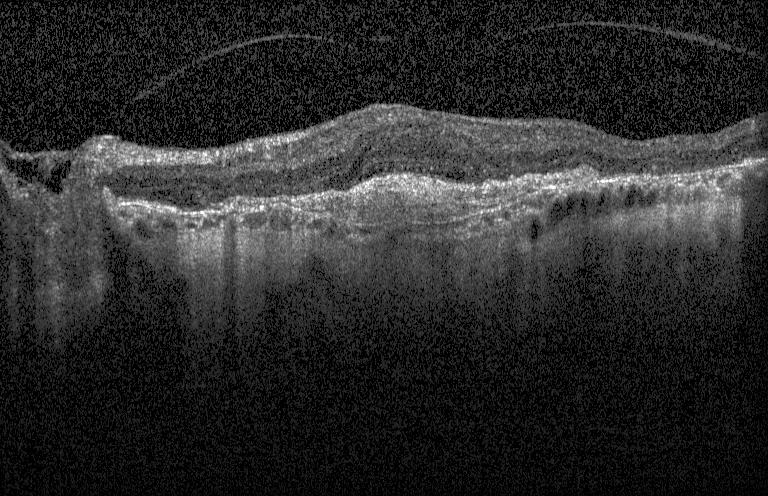 Optical coherence tomography B-scan. OCT finding: choroidal neovascularization.